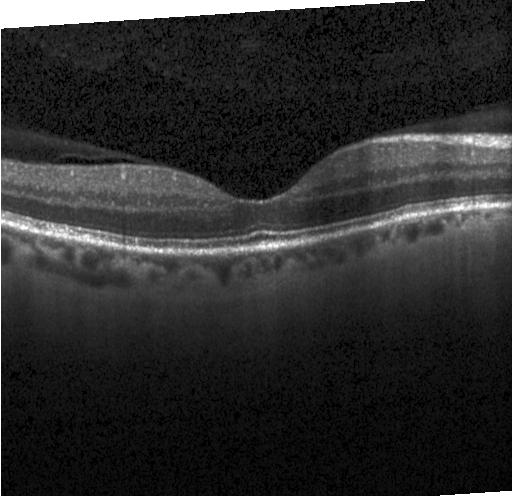 OCT B-scan showing no CNV, no DME, and no drusen.